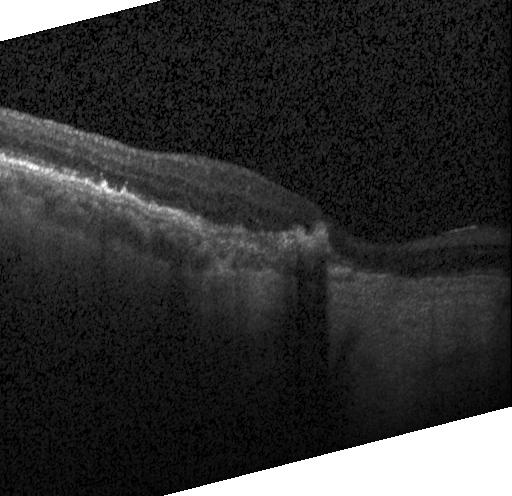
Acquired on a Heidelberg Spectralis · spectral-domain optical coherence tomography · fovea-centered · optical coherence tomography scan — OCT finding: CNV.